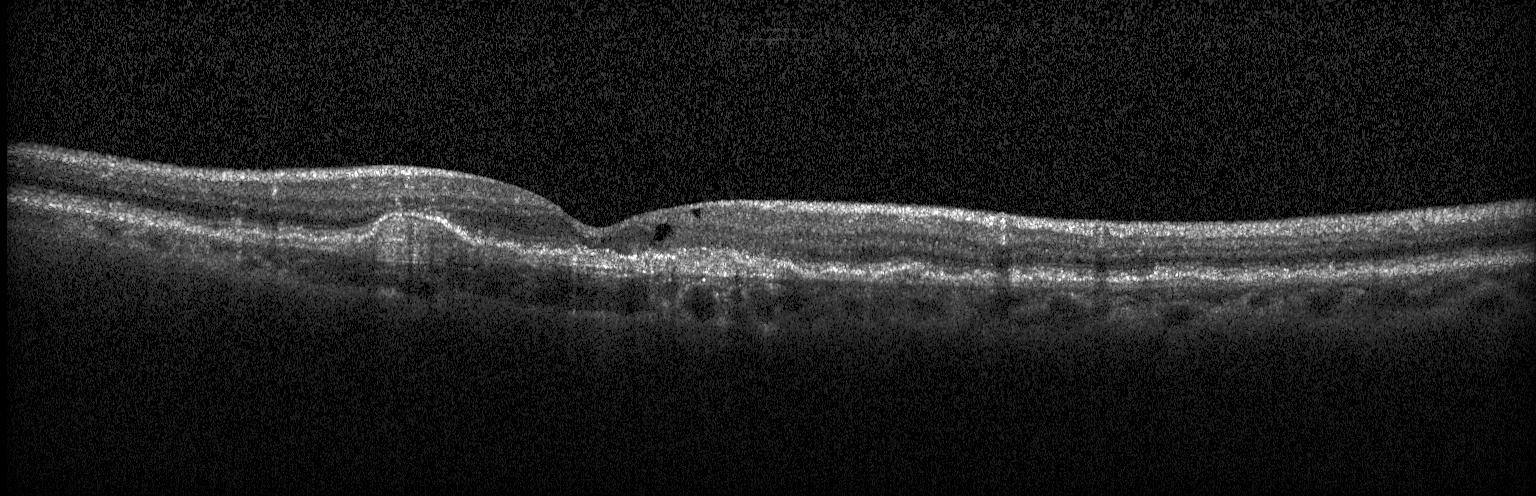 Heidelberg Spectralis OCT system · retinal OCT B-scan · spectral-domain optical coherence tomography · horizontal scan through the fovea — Impression: choroidal neovascularization (CNV).